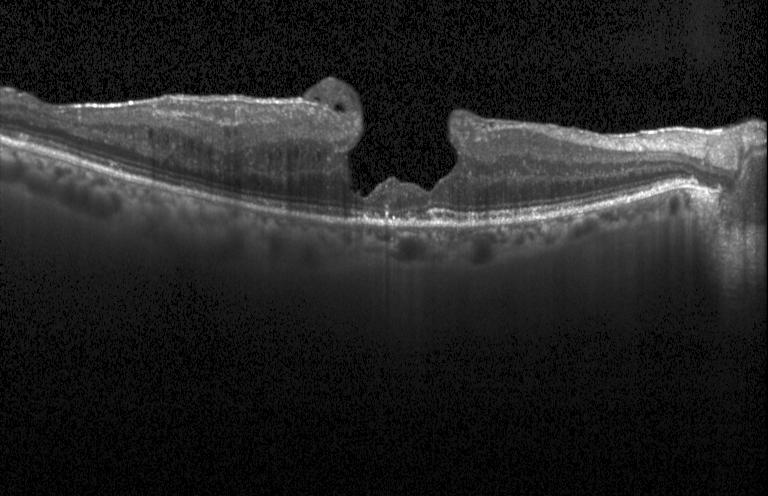 Assessment: diabetic macular edema.